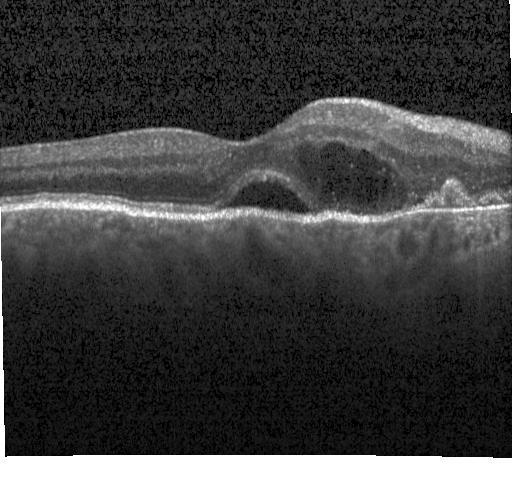

Horizontal scan through the fovea · optical coherence tomography scan · acquired on a Heidelberg Spectralis — Macular OCT: a choroidal neovascular membrane.